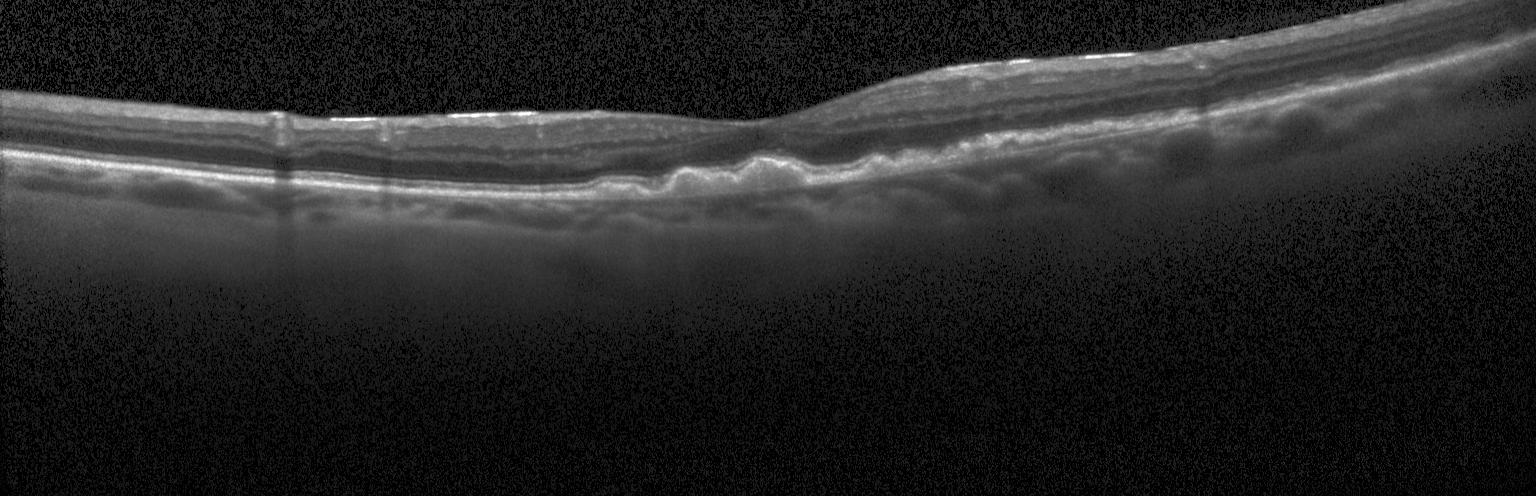 OCT B-scan.
This B-scan demonstrates sub-RPE drusenoid deposits.